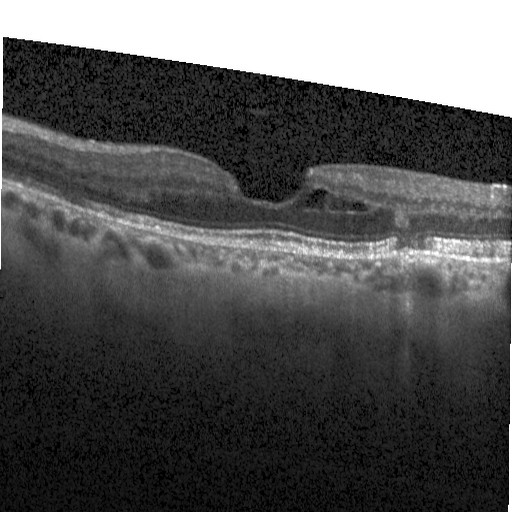 Finding: diabetic macular edema.